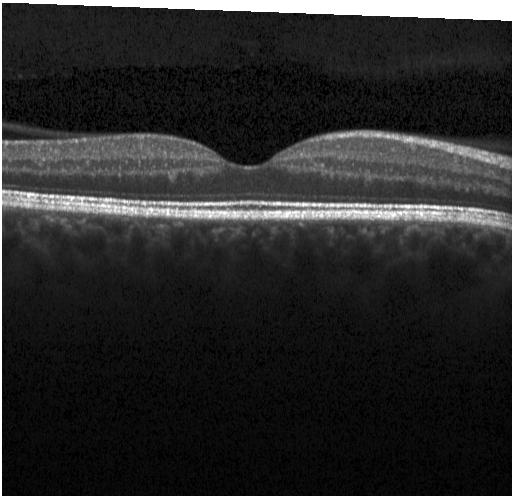
Macular OCT: no evidence of CNV, DME, or drusen.